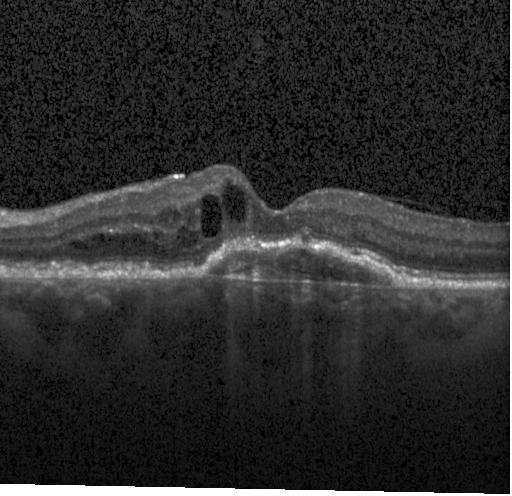
Instrument: Heidelberg Spectralis, through the macula, retinal OCT cross-section, SD-OCT. The scan shows CNV.